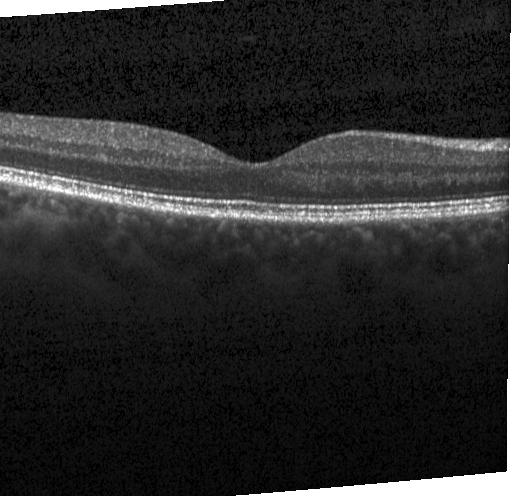 Retinal OCT B-scan, Heidelberg Spectralis. Diagnosis: no choroidal neovascularization, diabetic macular edema, or drusen.